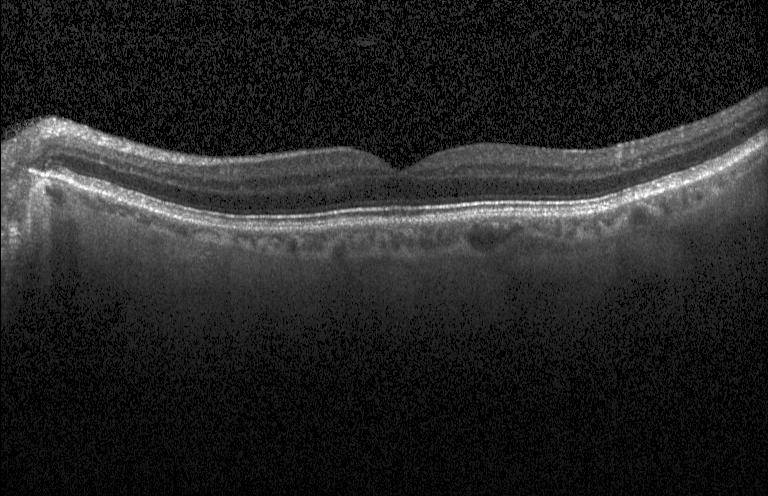

OCT scan showing no choroidal neovascularization, diabetic macular edema, or drusen.